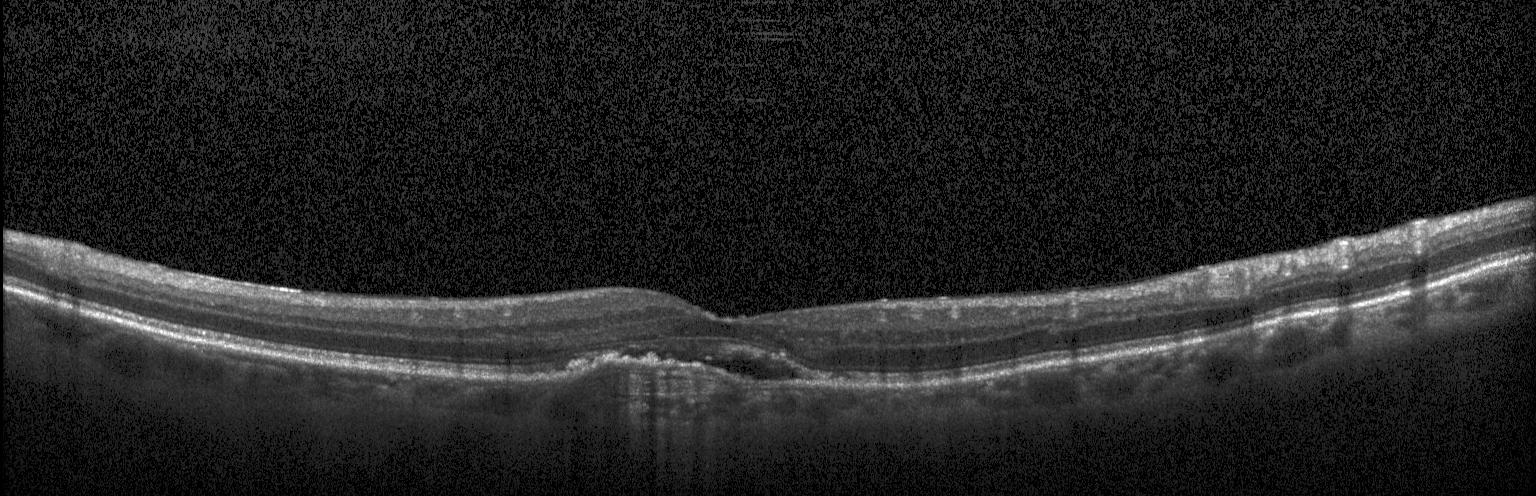
Diagnosis: a choroidal neovascular membrane.